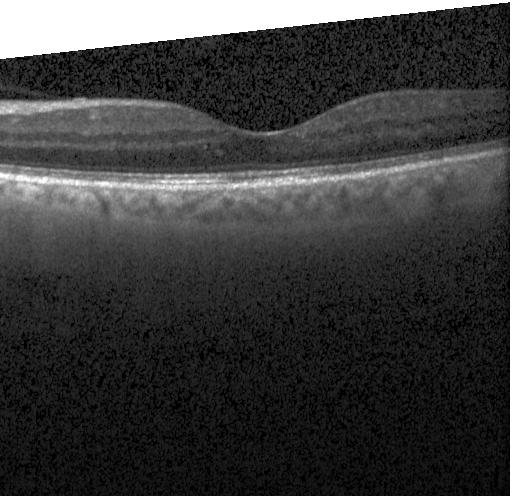
OCT B-scan.
This B-scan demonstrates no evidence of CNV, DME, or drusen.